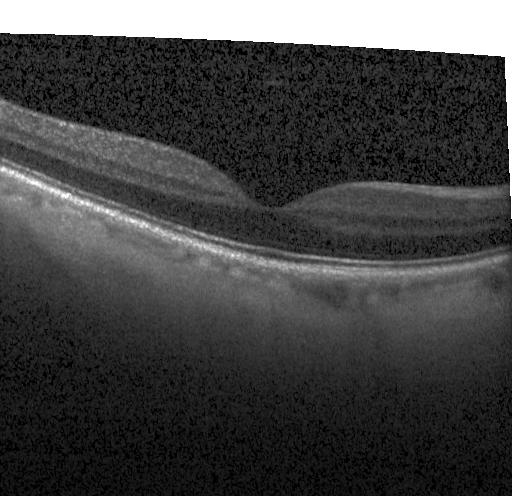
Acquired on a Heidelberg Spectralis; OCT line scan; spectral-domain OCT; fovea-centered. Assessment: neither choroidal neovascularization, diabetic macular edema, nor drusen.